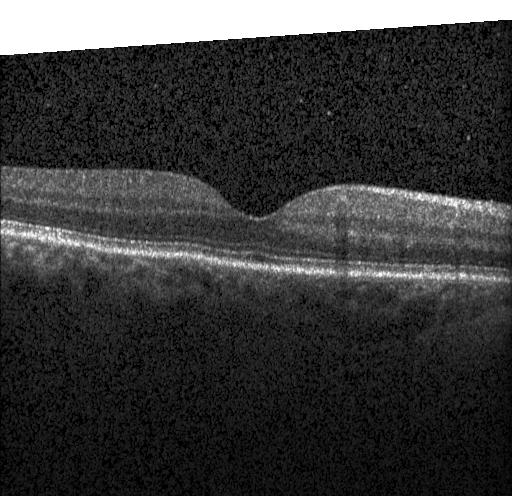
Dx: no evidence of choroidal neovascularization, diabetic macular edema, or drusen.